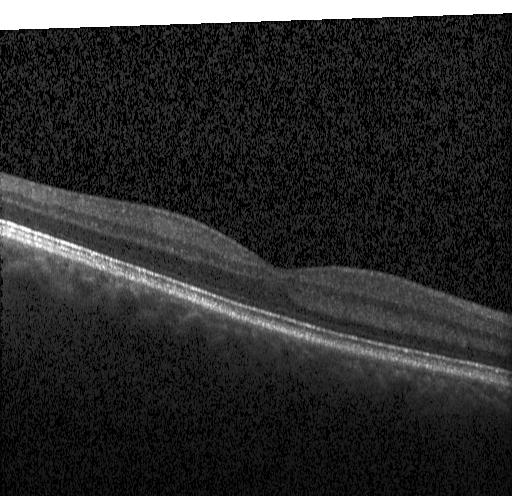 Optical coherence tomography scan. Finding: no choroidal neovascularization, diabetic macular edema, or drusen.